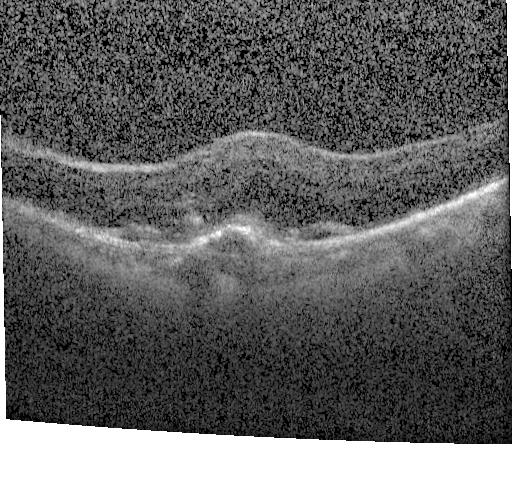
Diagnosis: CNV.